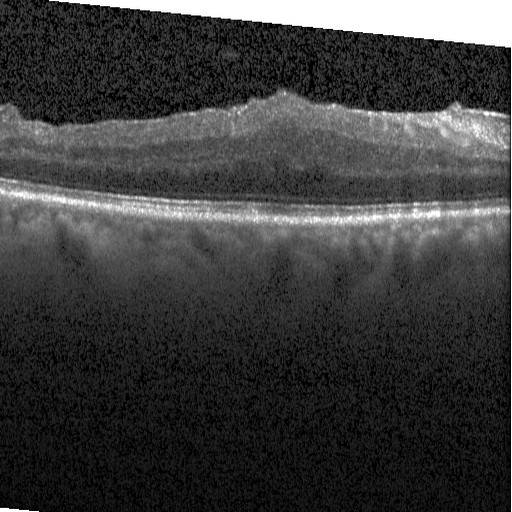
Macular OCT demonstrating diabetic macular edema.